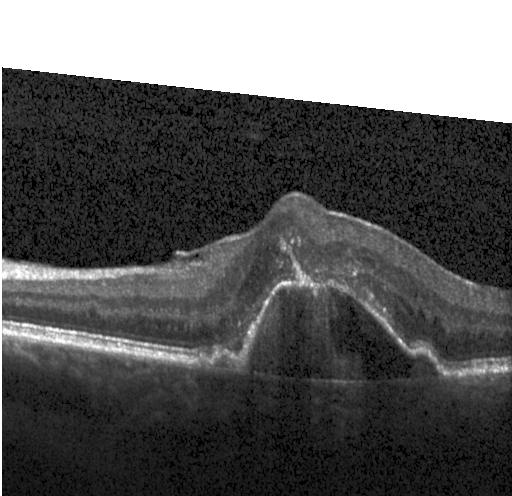
Assessment: a choroidal neovascular membrane.